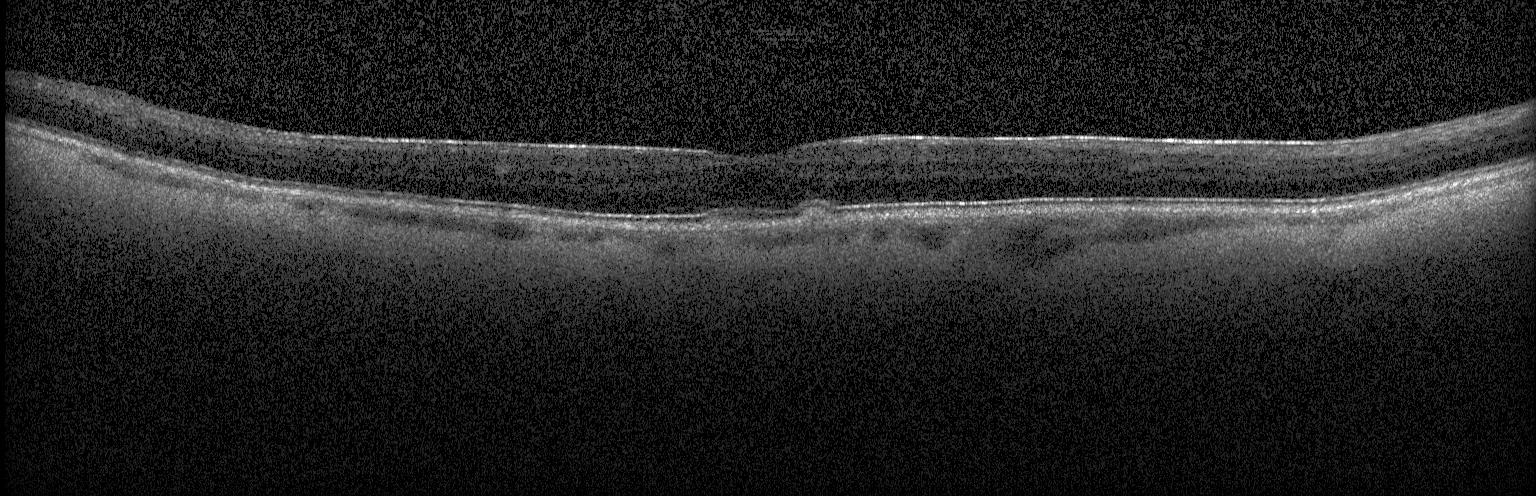
Impression: multiple drusen.